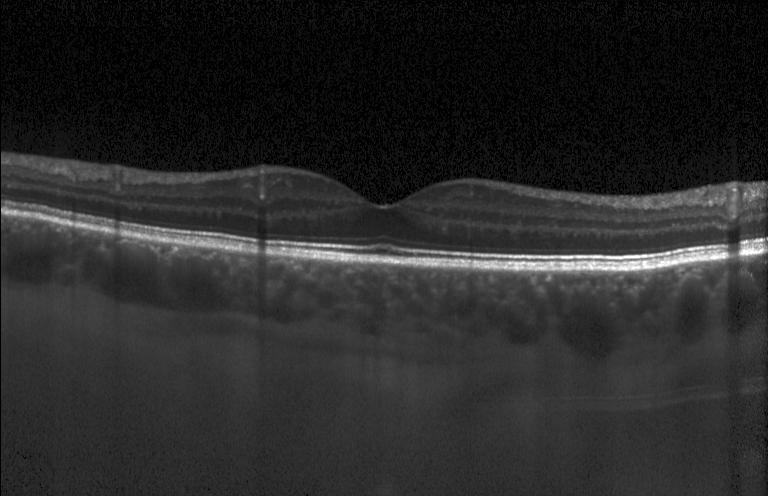

Spectral-domain optical coherence tomography · retinal OCT cross-section
Finding: no choroidal neovascularization, diabetic macular edema, or drusen.